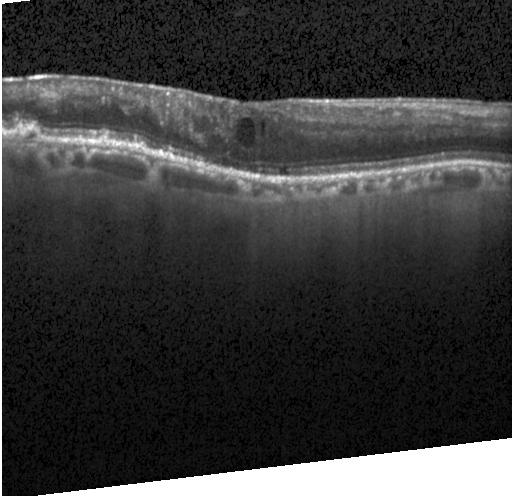 OCT line scan — Finding: choroidal neovascularization.